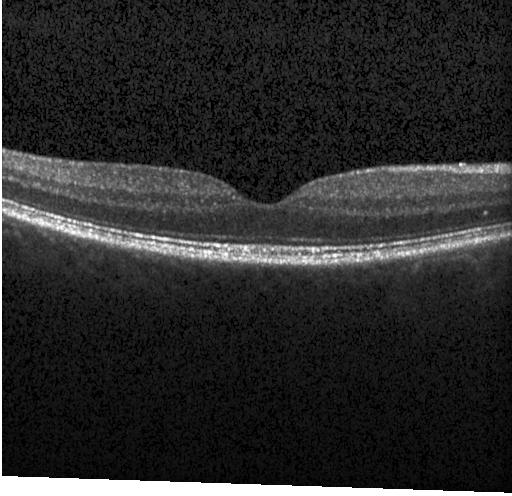
OCT scan showing no evidence of choroidal neovascularization, diabetic macular edema, or drusen.